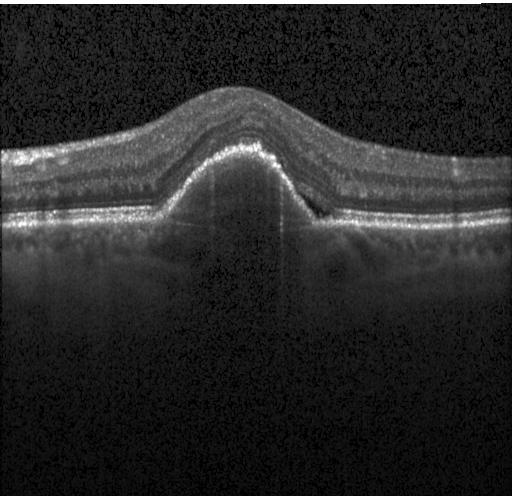
Optical coherence tomography scan.
This B-scan demonstrates choroidal neovascularization.